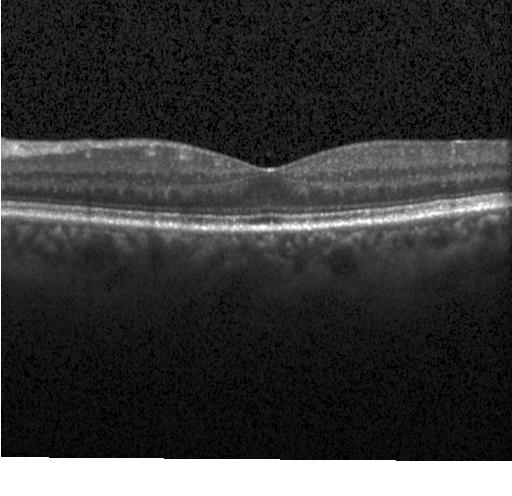

The scan shows no choroidal neovascularization, no diabetic macular edema, and no drusen.